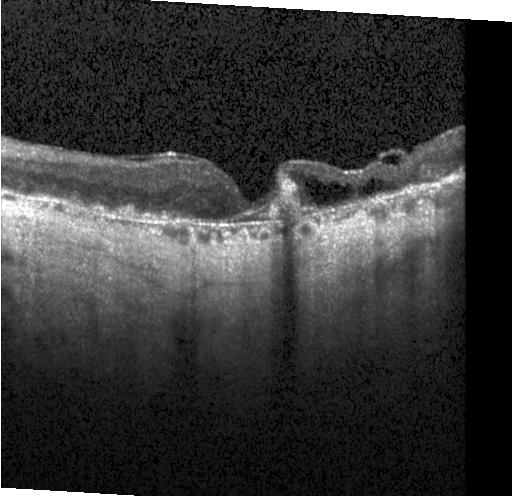
Through the macula, retinal OCT B-scan, spectral-domain optical coherence tomography, instrument: Heidelberg Spectralis — Macular OCT: choroidal neovascularization.